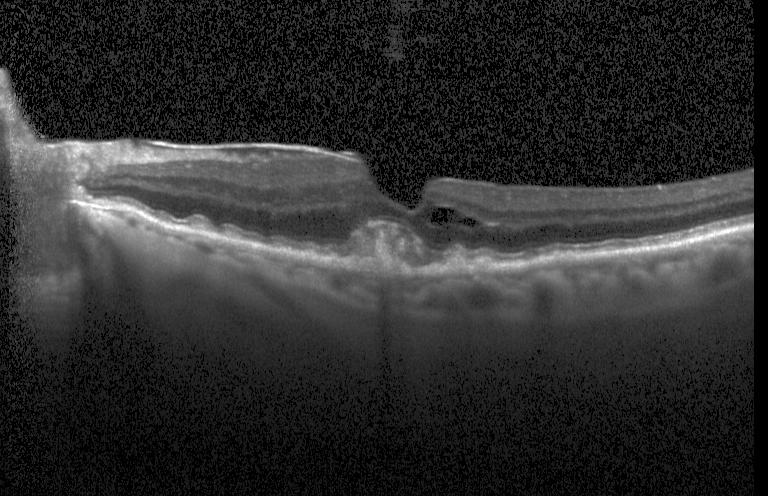

Spectral-domain OCT. OCT line scan. Horizontal scan through the fovea
Diagnosis: a choroidal neovascular membrane.